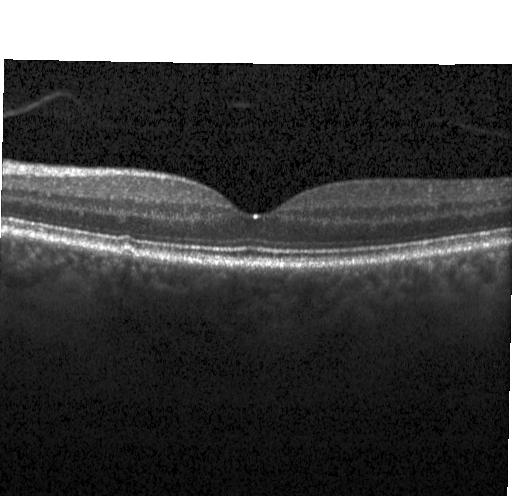
Sub-RPE drusenoid deposits.